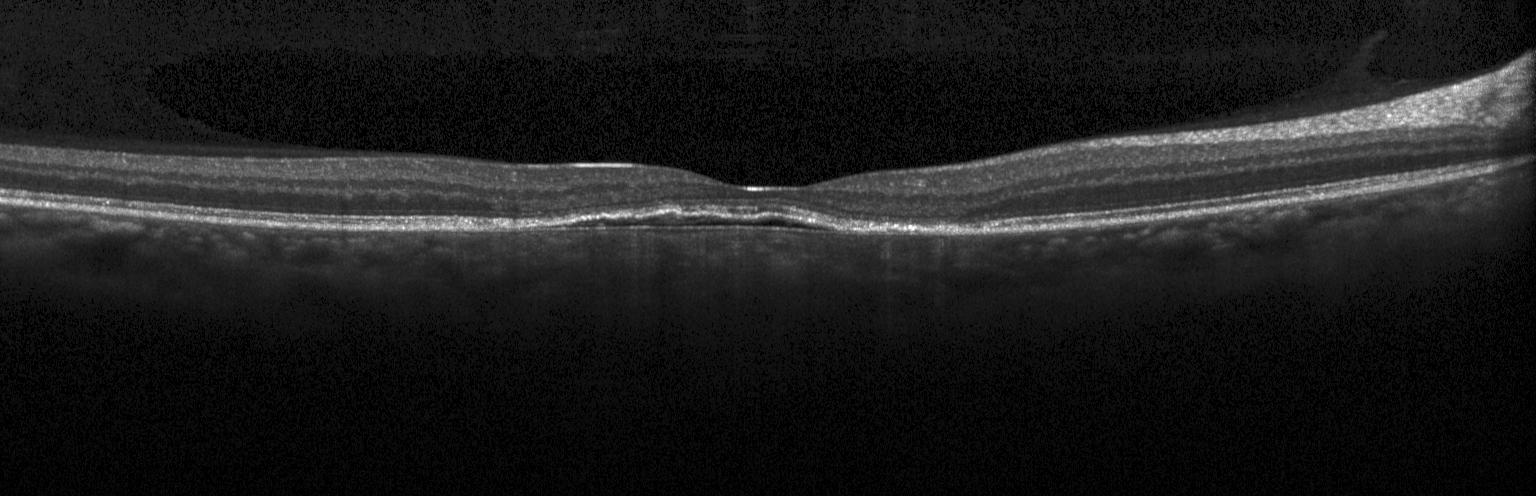

OCT line scan. Spectral-domain optical coherence tomography. Instrument: Heidelberg Spectralis — Assessment: a choroidal neovascular membrane.